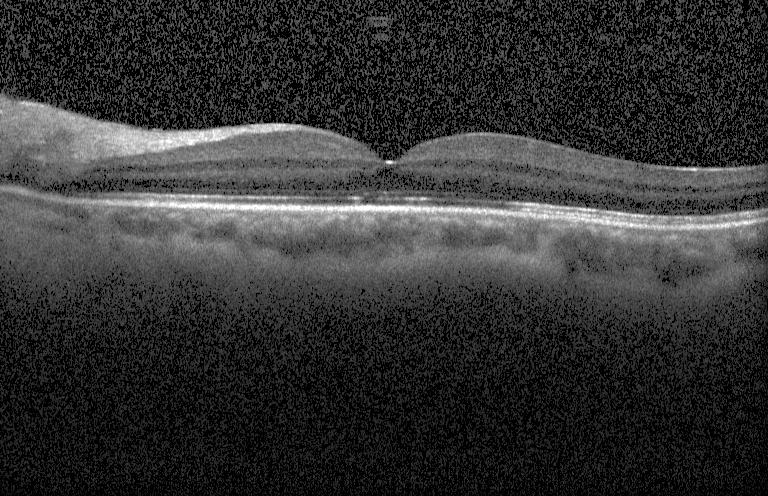

Assessment: no evidence of choroidal neovascularization, diabetic macular edema, or drusen.